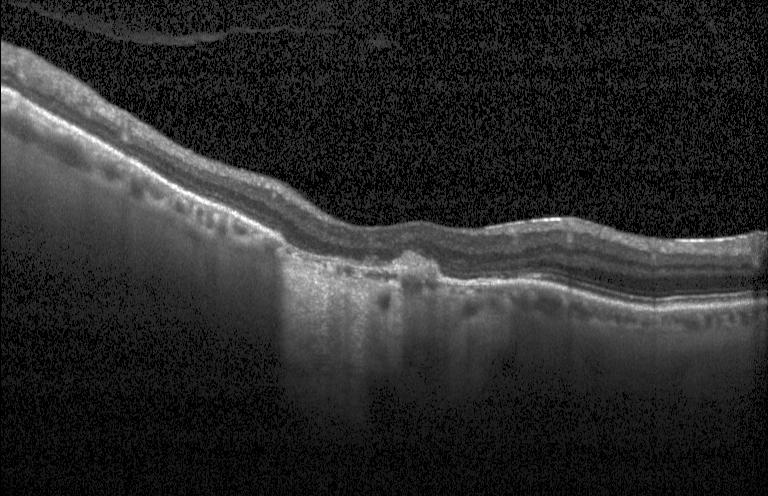
OCT scan showing a choroidal neovascular membrane.